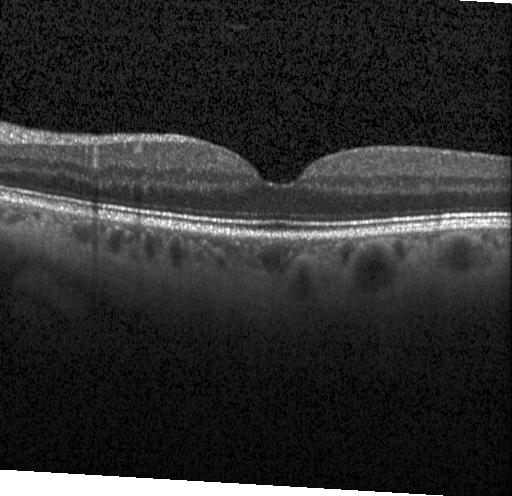
Diagnosis: no evidence of choroidal neovascularization, diabetic macular edema, or drusen.